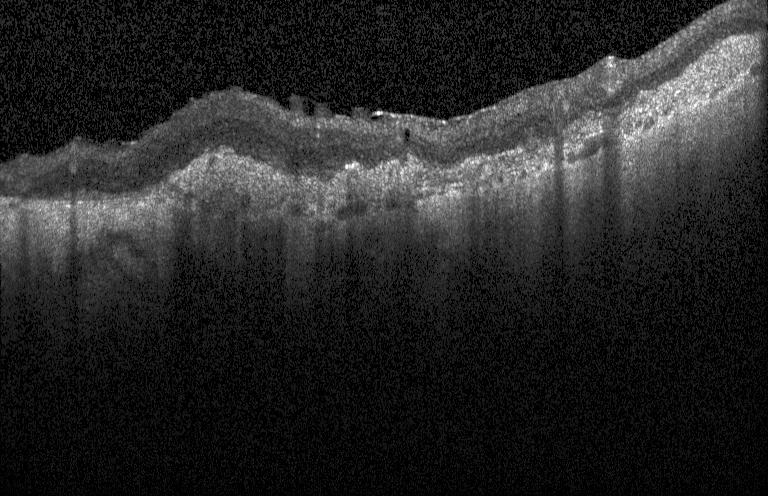
Spectral-domain optical coherence tomography; acquired on a Heidelberg Spectralis; retinal OCT B-scan; through the macula. A choroidal neovascular membrane.